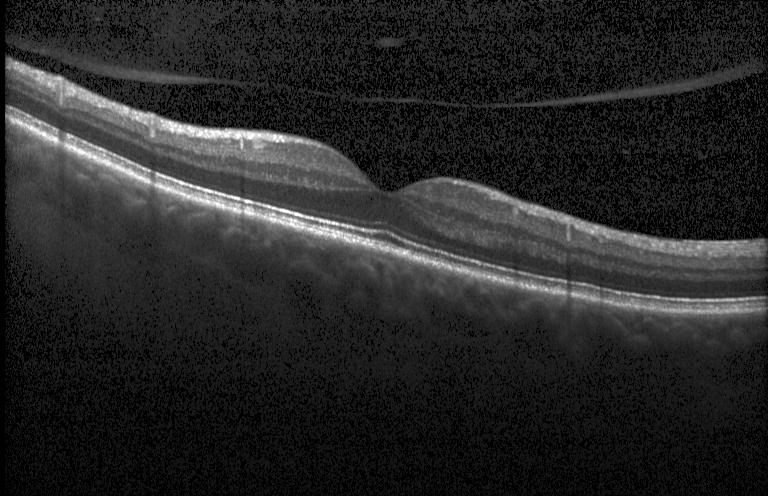
Spectral-domain OCT. Retinal OCT cross-section. Horizontal scan through the fovea — The scan shows no evidence of choroidal neovascularization, diabetic macular edema, or drusen.